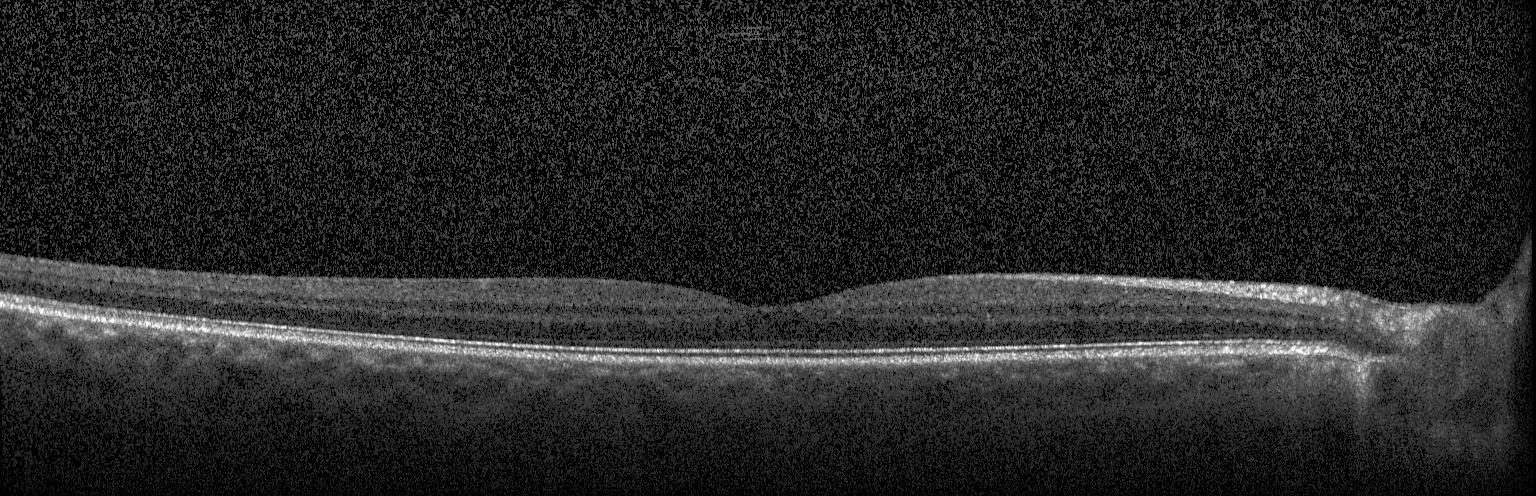 Optical coherence tomography B-scan; Heidelberg Spectralis; spectral-domain OCT; fovea-centered. Impression: neither CNV, DME, nor drusen.